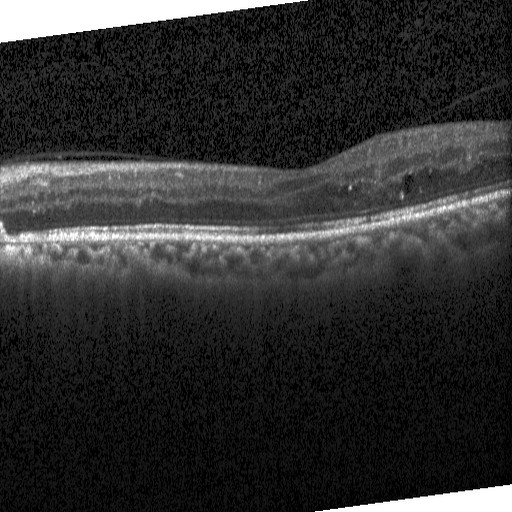

OCT B-scan. Fovea-centered. Instrument: Heidelberg Spectralis. SD-OCT. Impression: diabetic macular edema (DME).